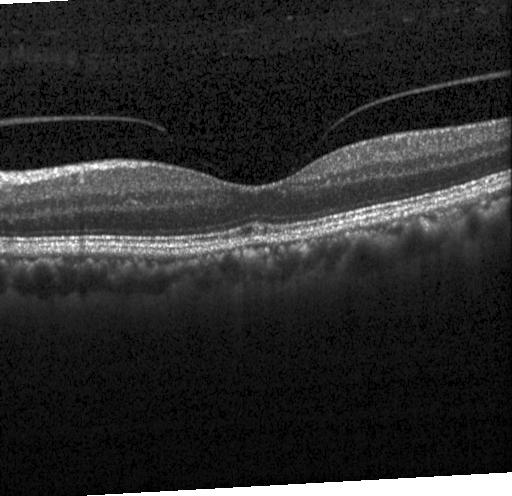
Optical coherence tomography B-scan — Impression: no evidence of choroidal neovascularization, diabetic macular edema, or drusen.